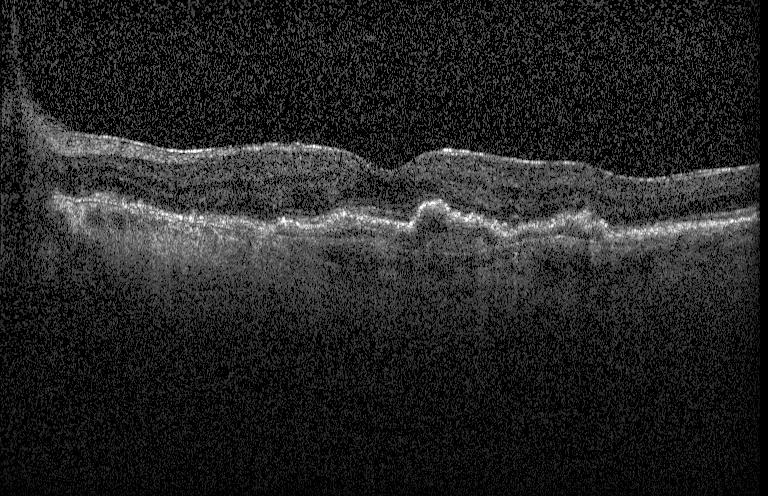

OCT line scan · SD-OCT · acquired on a Heidelberg Spectralis · centered on the fovea. Choroidal neovascularization.